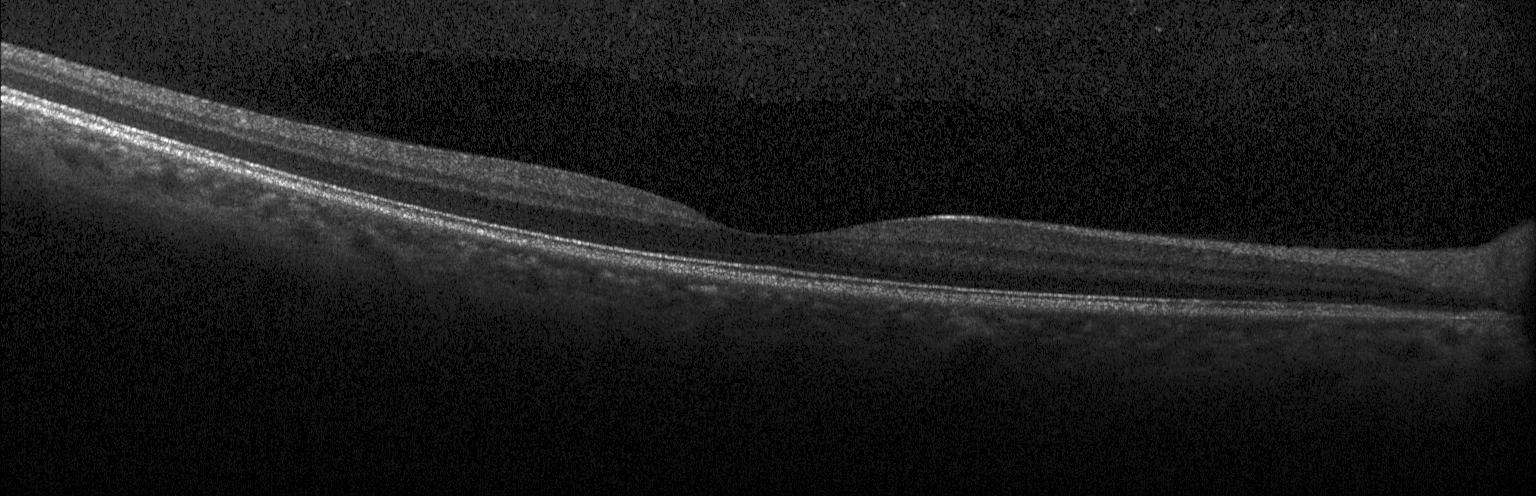 This B-scan demonstrates no evidence of CNV, DME, or drusen.